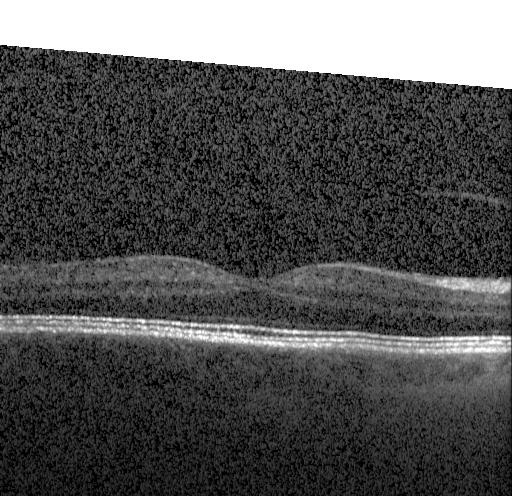
Spectral-domain OCT B-scan: no choroidal neovascularization, diabetic macular edema, or drusen.